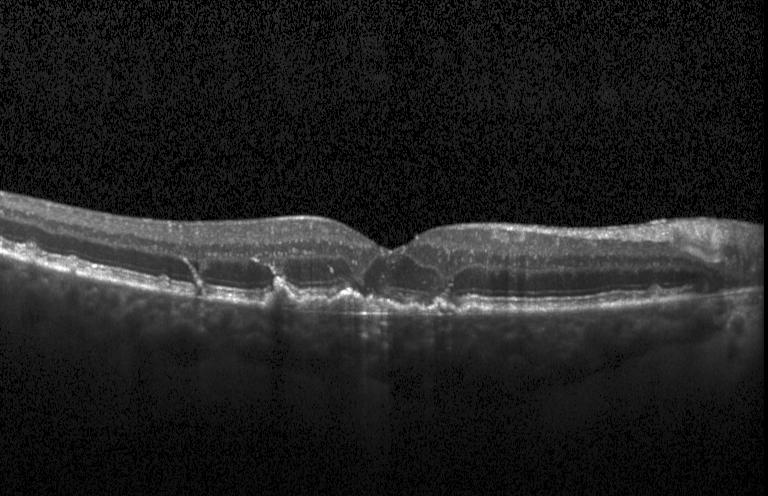 Optical coherence tomography scan.
Diagnosis: a choroidal neovascular membrane.